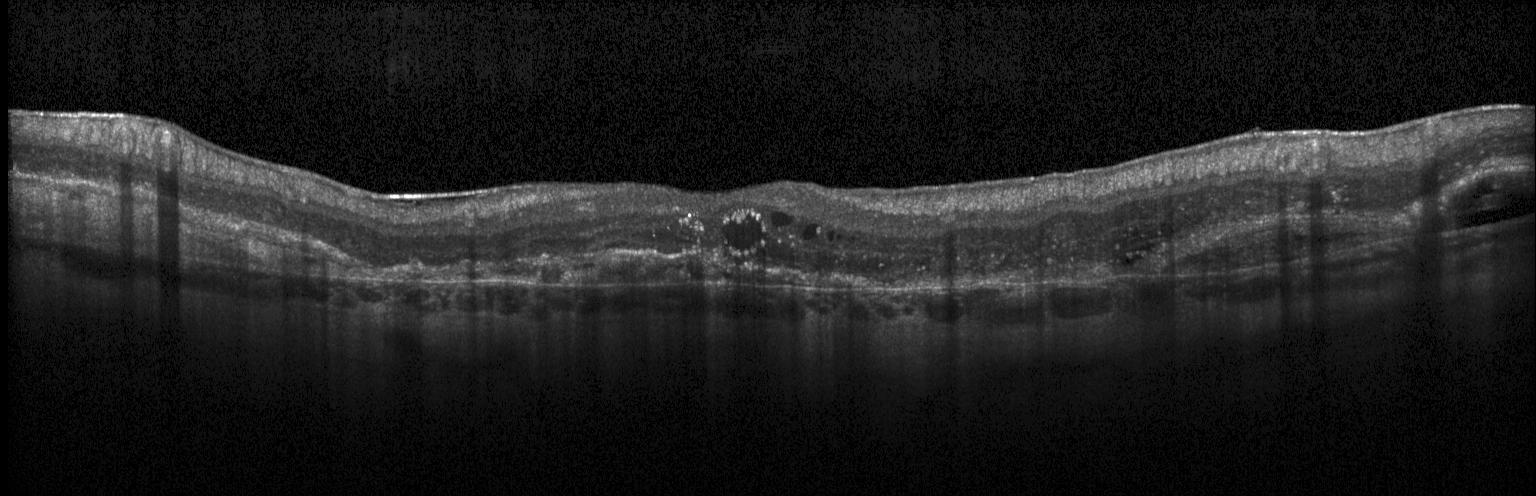

Optical coherence tomography scan · SD-OCT
Finding: a choroidal neovascular membrane.